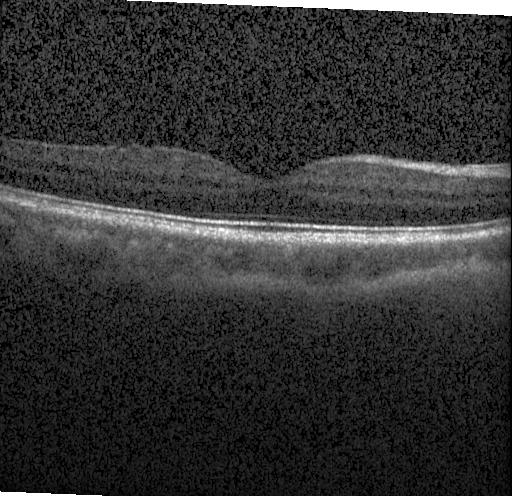

Through the macula; SD-OCT; acquired on a Heidelberg Spectralis; retinal OCT B-scan — OCT finding: no evidence of choroidal neovascularization, diabetic macular edema, or drusen.